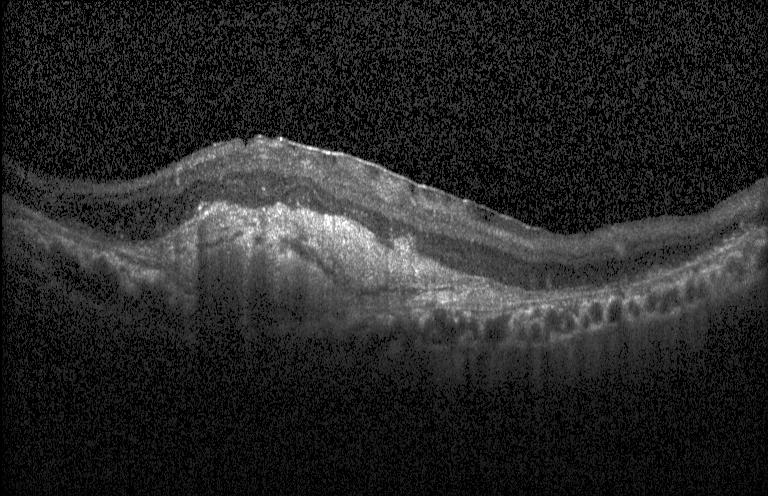

Spectral-domain OCT · OCT line scan.
Macular OCT: a choroidal neovascular membrane.